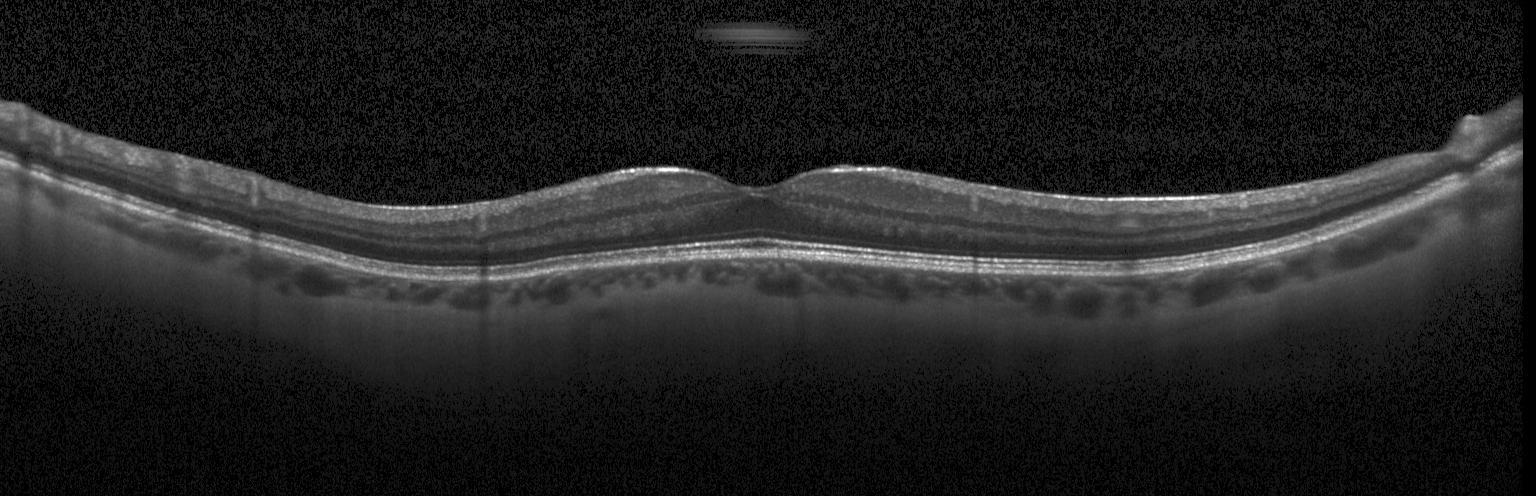 Heidelberg Spectralis. OCT B-scan.
Finding: no choroidal neovascularization, diabetic macular edema, or drusen.